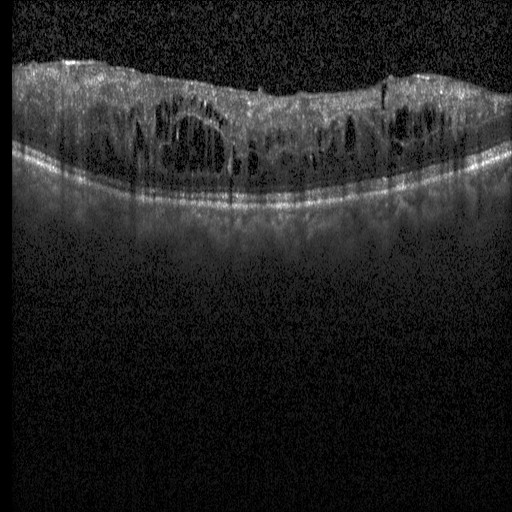 Spectral-domain optical coherence tomography, acquired on a Heidelberg Spectralis, horizontal scan through the fovea, optical coherence tomography scan
Macular OCT: diabetic macular edema.